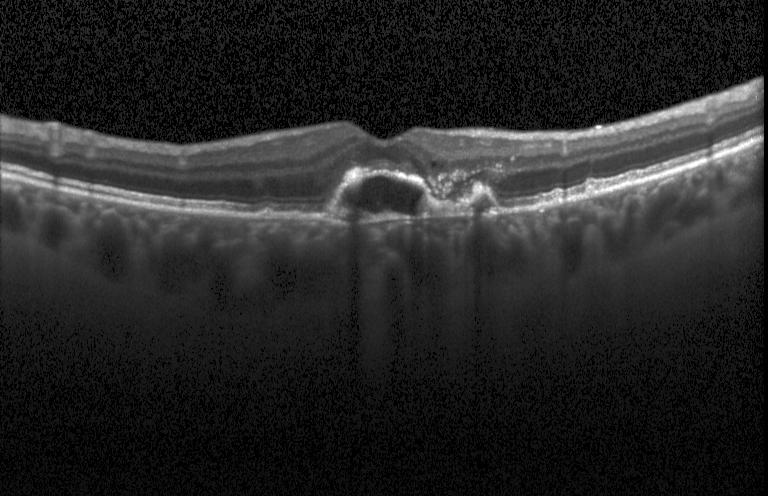

Diagnosis: a choroidal neovascular membrane.